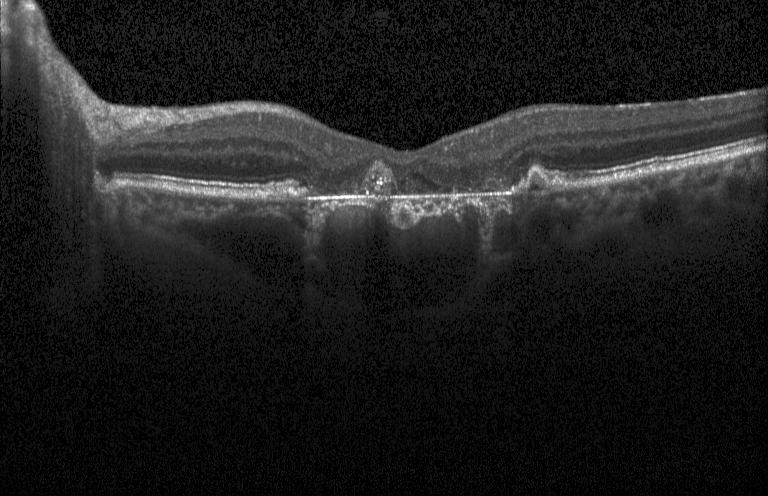 Retinal OCT cross-section · fovea-centered. Impression: choroidal neovascularization (CNV).